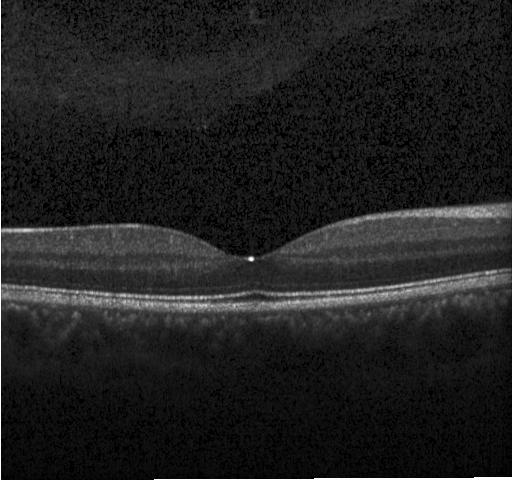
OCT line scan
The scan shows no choroidal neovascularization, no diabetic macular edema, and no drusen.